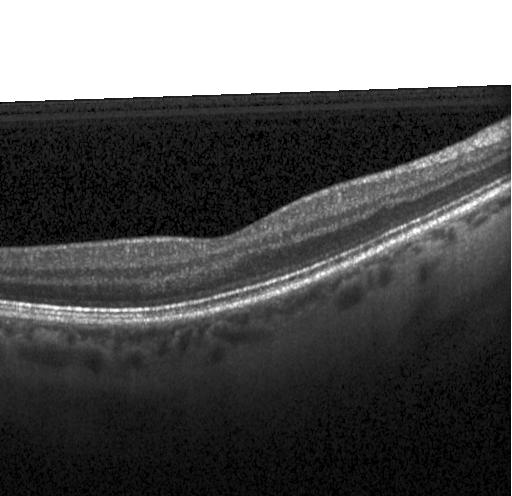

Instrument: Heidelberg Spectralis. Through the macula. Retinal OCT cross-section. SD-OCT — Finding: no evidence of choroidal neovascularization, diabetic macular edema, or drusen.